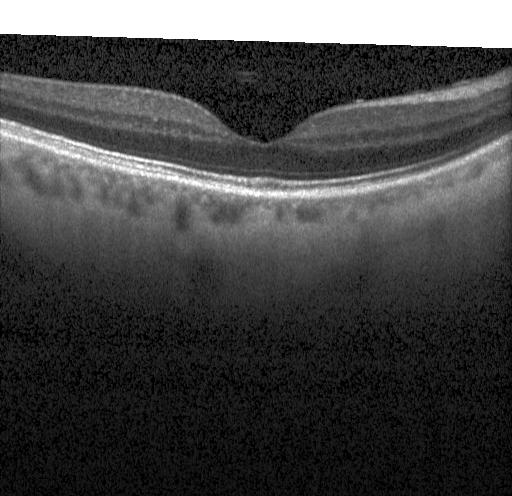

Retinal OCT cross-section.
Assessment: no choroidal neovascularization, diabetic macular edema, or drusen.